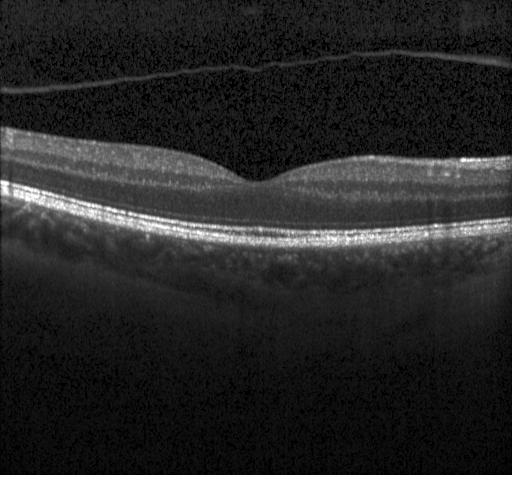 Retinal OCT B-scan
The scan shows no choroidal neovascularization, diabetic macular edema, or drusen.